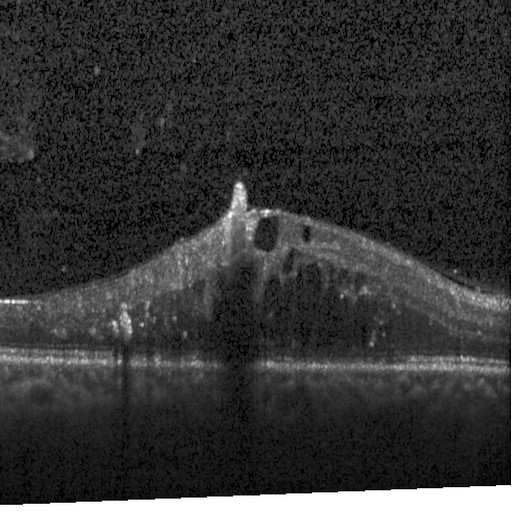 SD-OCT · acquired on a Heidelberg Spectralis · OCT line scan. Dx: DME.